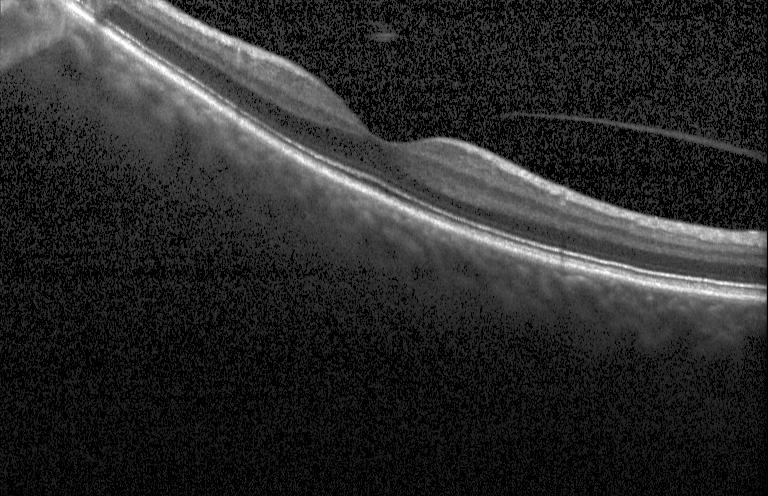

Assessment: no CNV, DME, or drusen.